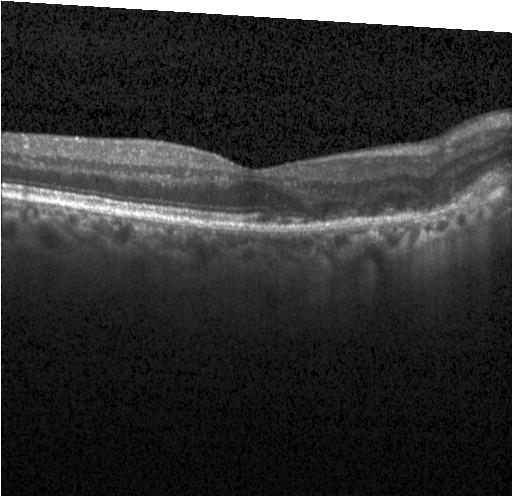

Spectral-domain optical coherence tomography; optical coherence tomography scan; macular scan
This B-scan demonstrates a choroidal neovascular membrane.